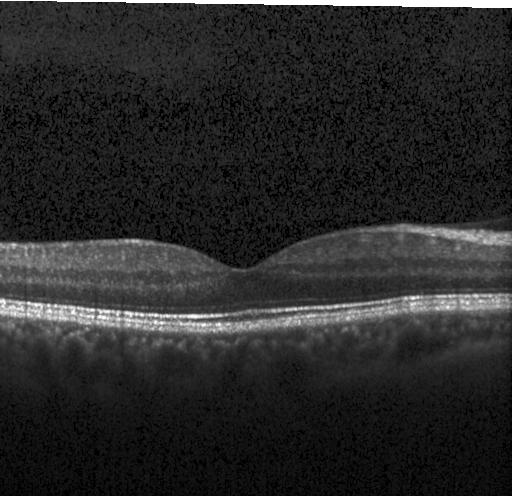

Retinal OCT B-scan, centered on the fovea — Finding: neither choroidal neovascularization, diabetic macular edema, nor drusen.